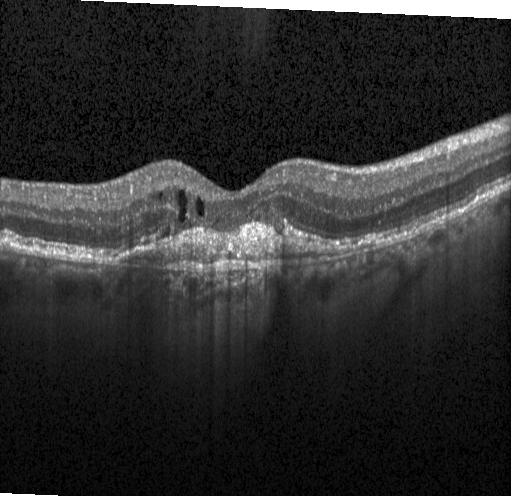
Optical coherence tomography B-scan — Diagnosis: a choroidal neovascular membrane.